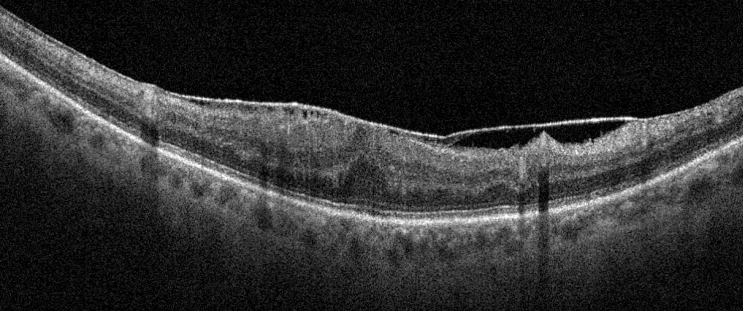 Retinal OCT B-scan, Optovue Avanti RTVue XR, through the macula — Impression: ERM.